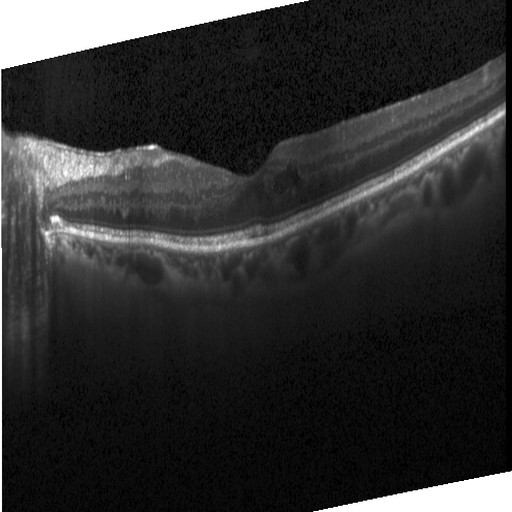 SD-OCT · optical coherence tomography scan · horizontal scan through the fovea. This B-scan demonstrates diabetic macular edema (DME).